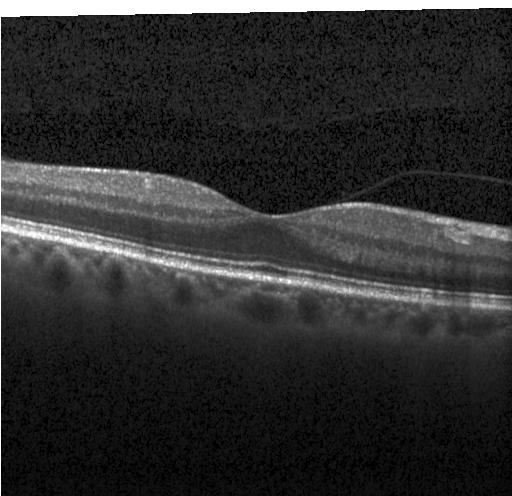

OCT line scan. Diagnosis: no choroidal neovascularization, no diabetic macular edema, and no drusen.